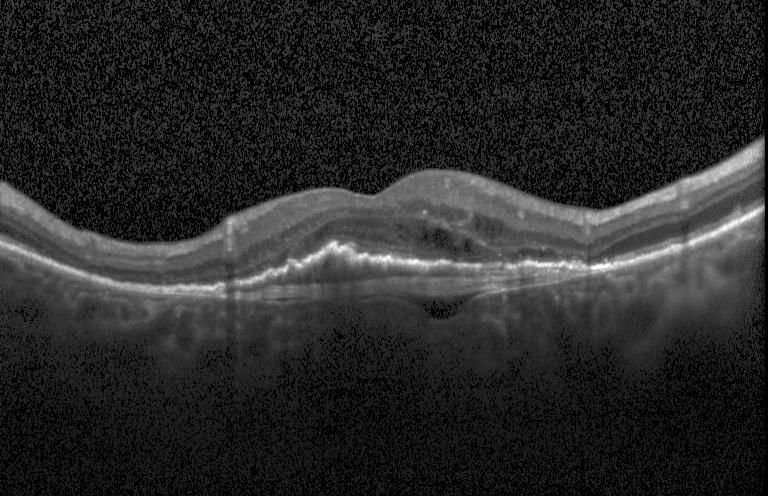
OCT B-scan showing choroidal neovascularization.